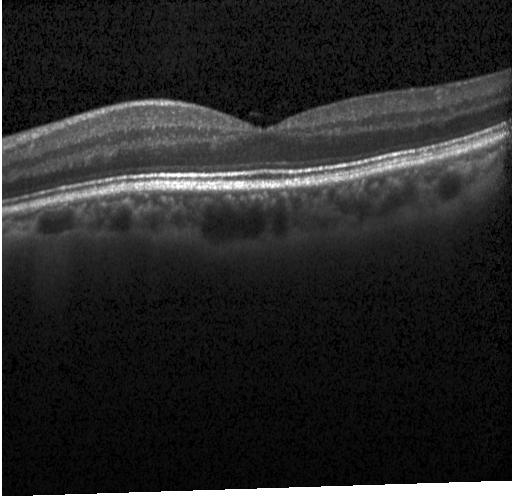 Retinal OCT cross-section showing neither CNV, DME, nor drusen.